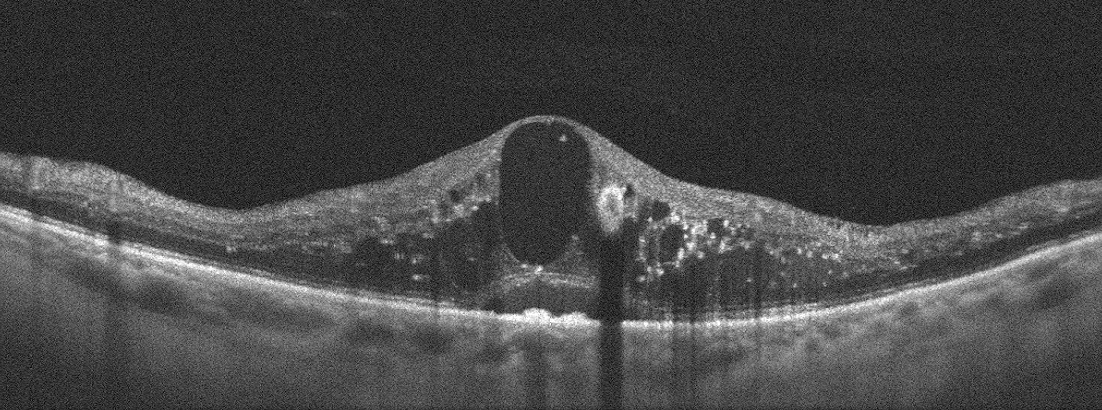 Dx: diabetic macular edema.